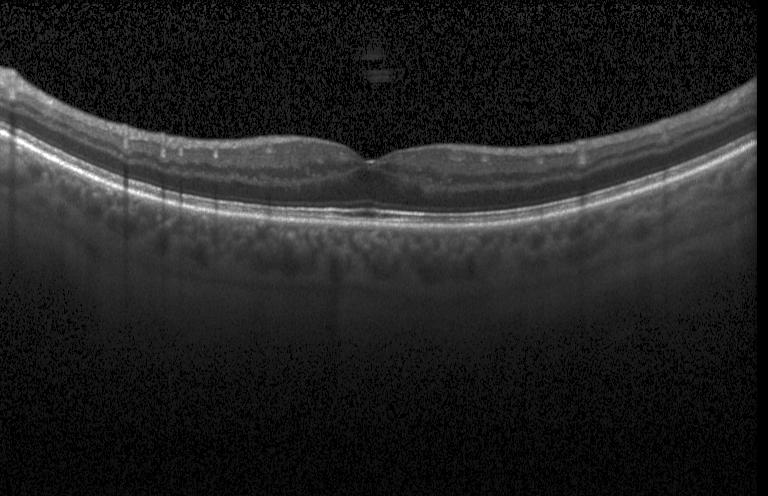
Heidelberg Spectralis · horizontal scan through the fovea · spectral-domain optical coherence tomography · OCT line scan
Macular OCT: neither CNV, DME, nor drusen.